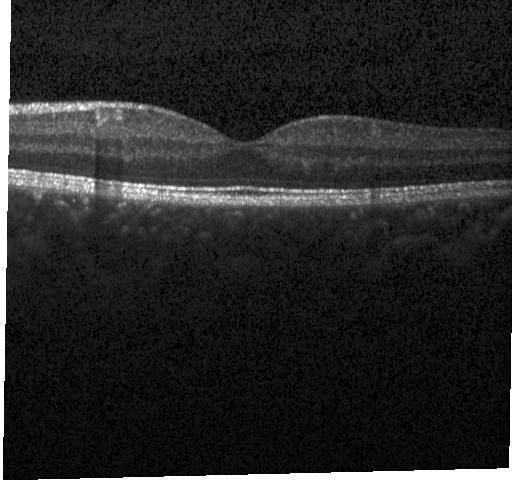
OCT B-scan — Finding: no choroidal neovascularization, no diabetic macular edema, and no drusen.